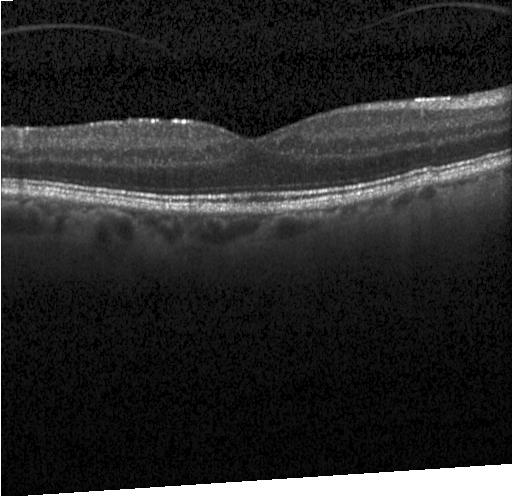

Finding: no CNV, DME, or drusen.